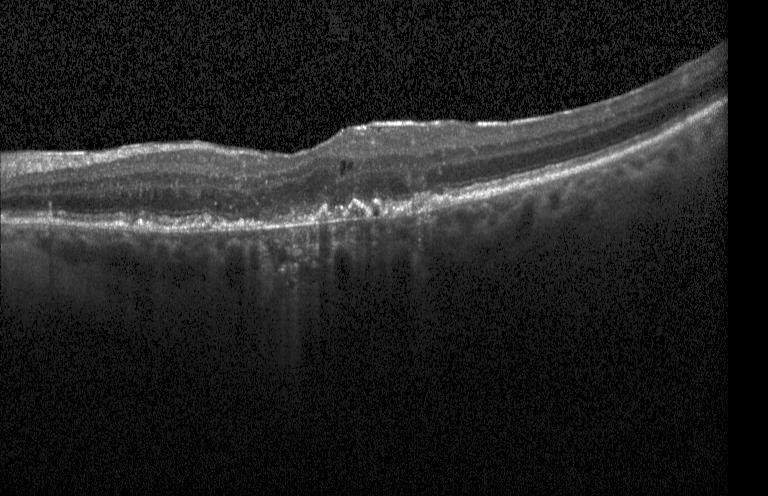 Spectral-domain OCT. Heidelberg Spectralis OCT system. Optical coherence tomography B-scan. Through the macula — Impression: a choroidal neovascular membrane.